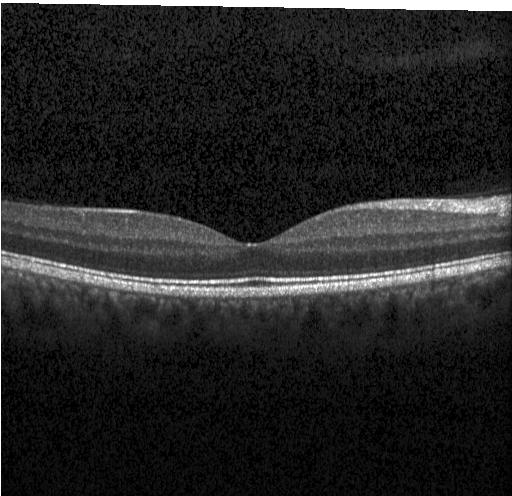
Impression: neither choroidal neovascularization, diabetic macular edema, nor drusen.